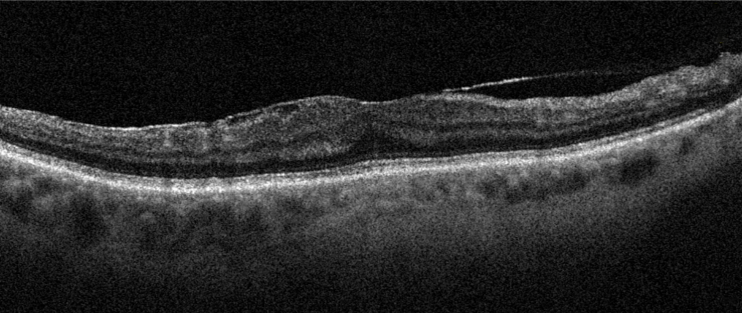

Fovea-centered. Retinal OCT cross-section. Optovue Avanti RTVue XR
The scan shows epiretinal membrane (ERM).